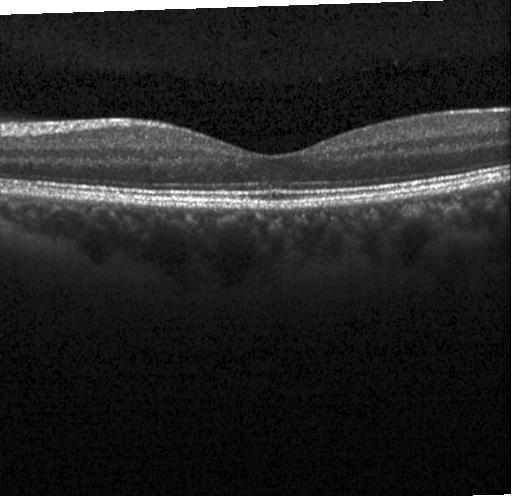
Diagnosis: no choroidal neovascularization, diabetic macular edema, or drusen.